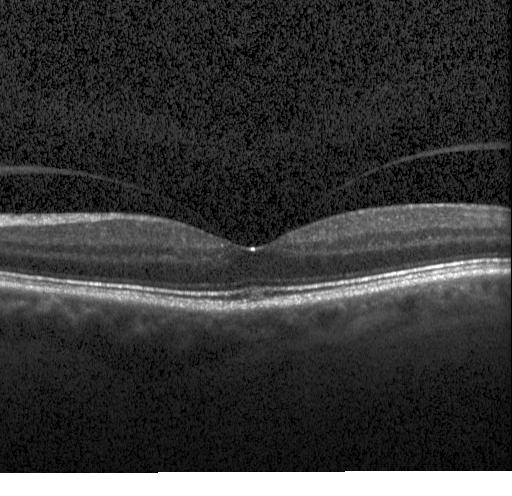 SD-OCT; optical coherence tomography B-scan.
Finding: no evidence of CNV, DME, or drusen.